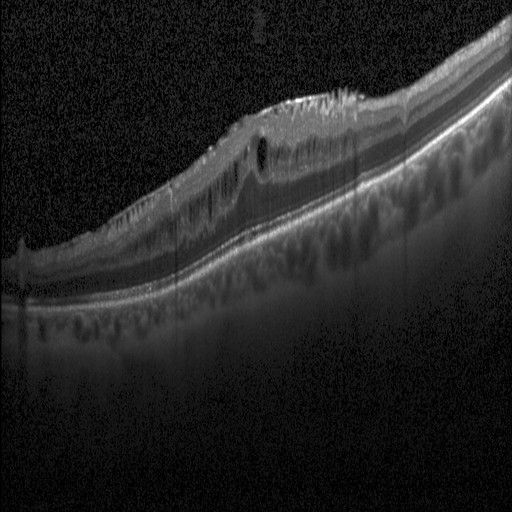
Retinal OCT cross-section showing diabetic macular edema.